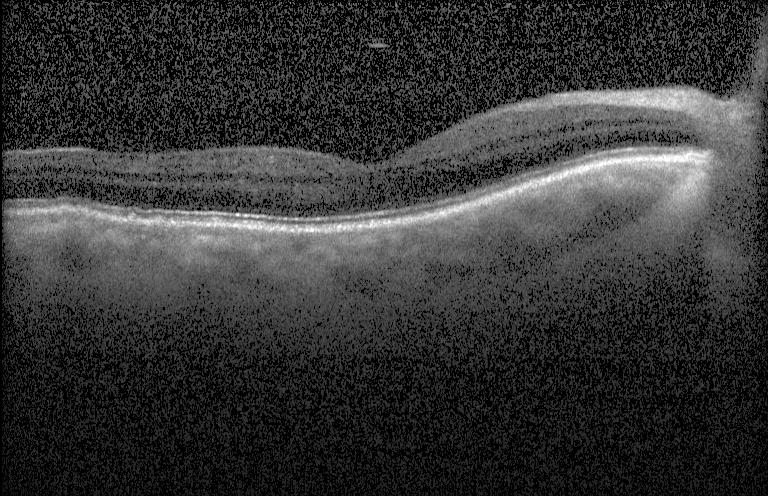

Optical coherence tomography scan. SD-OCT
Diagnosis: no choroidal neovascularization, diabetic macular edema, or drusen.